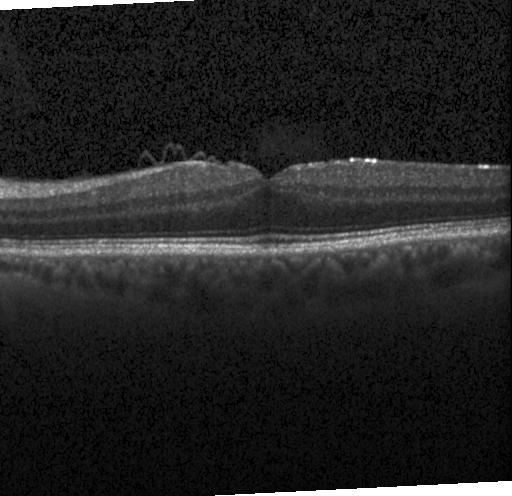
Centered on the fovea. Optical coherence tomography scan. Spectral-domain optical coherence tomography
Assessment: no CNV, DME, or drusen.